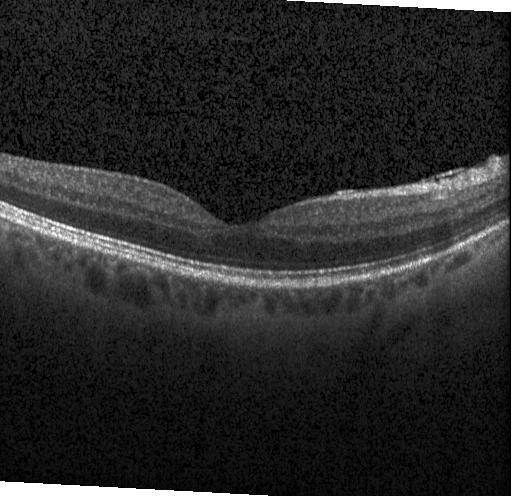
Acquired on a Heidelberg Spectralis · retinal OCT B-scan · fovea-centered
Finding: no CNV, no DME, and no drusen.